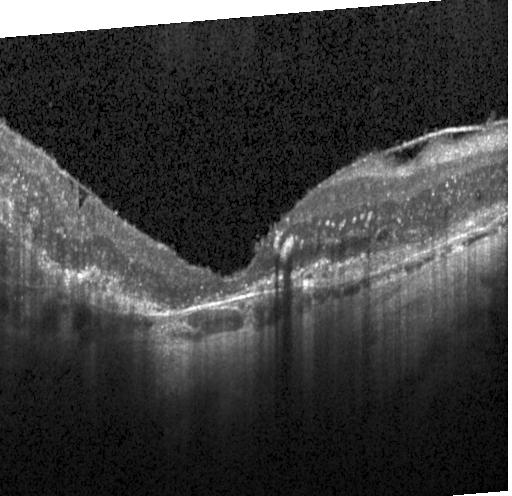
OCT finding: choroidal neovascularization (CNV).